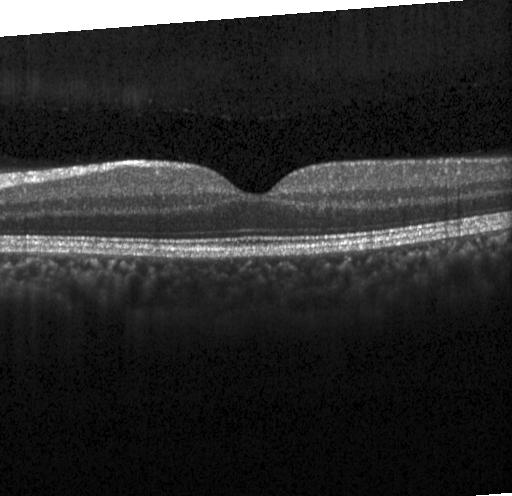

Through the macula. Retinal OCT cross-section. Instrument: Heidelberg Spectralis. Spectral-domain OCT.
This B-scan demonstrates no CNV, no DME, and no drusen.